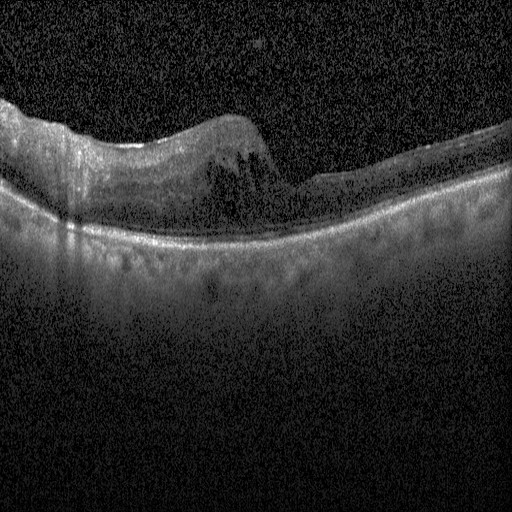
Retinal OCT B-scan · centered on the fovea · instrument: Heidelberg Spectralis
Finding: diabetic macular edema.